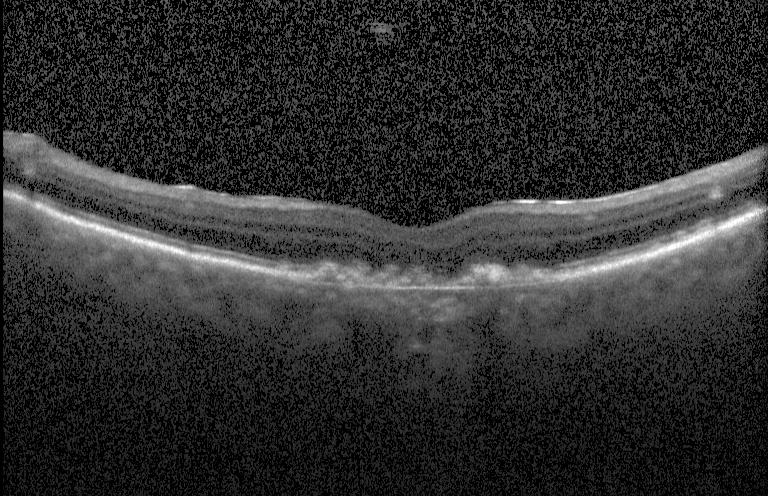 Assessment: a choroidal neovascular membrane.